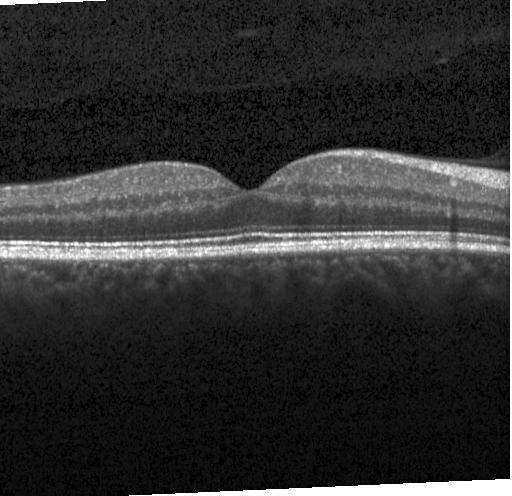
Impression: neither CNV, DME, nor drusen.